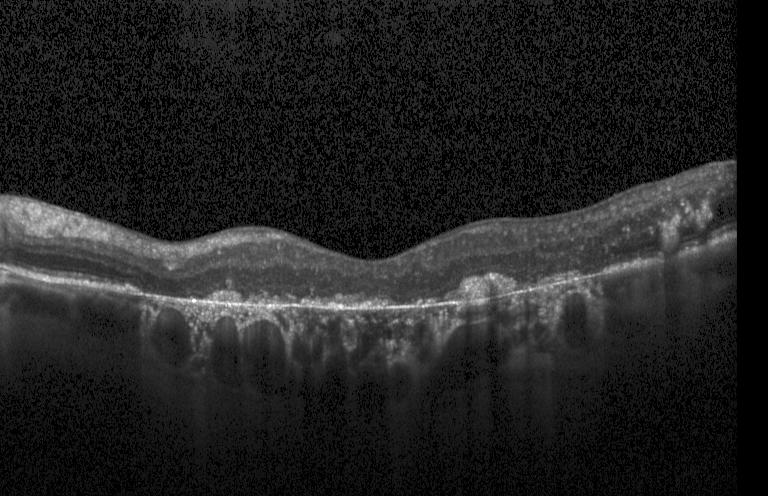 Optical coherence tomography scan.
Impression: a choroidal neovascular membrane.